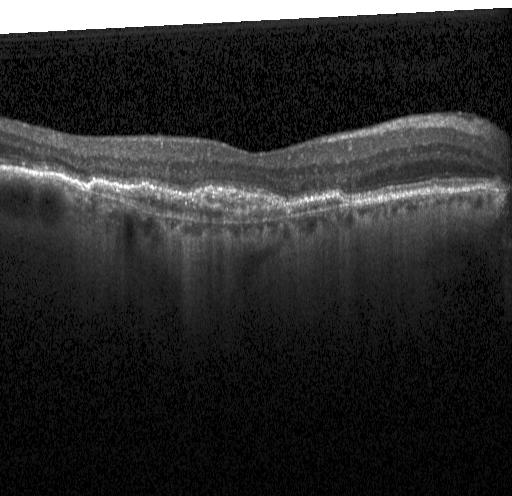
Retinal OCT B-scan; through the macula; Heidelberg Spectralis; SD-OCT — Diagnosis: a choroidal neovascular membrane.